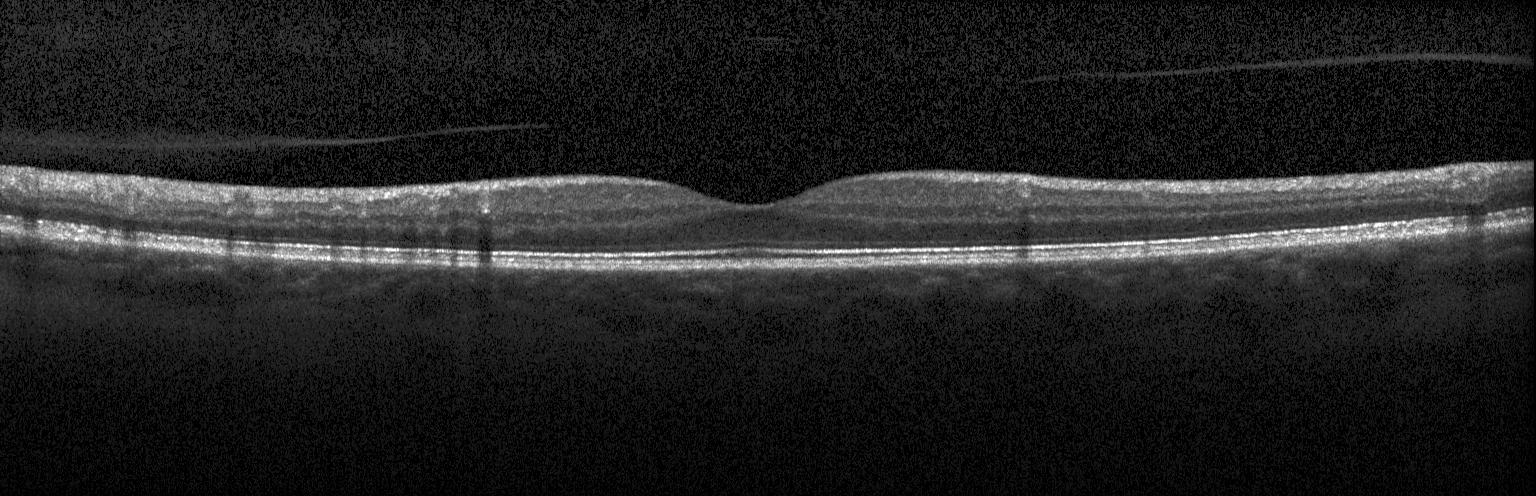 Horizontal scan through the fovea · SD-OCT · optical coherence tomography scan · Heidelberg Spectralis OCT system
OCT finding: no evidence of choroidal neovascularization, diabetic macular edema, or drusen.